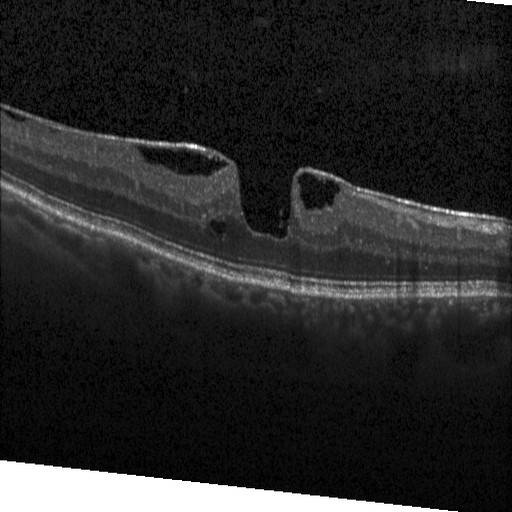 Finding: diabetic macular edema.